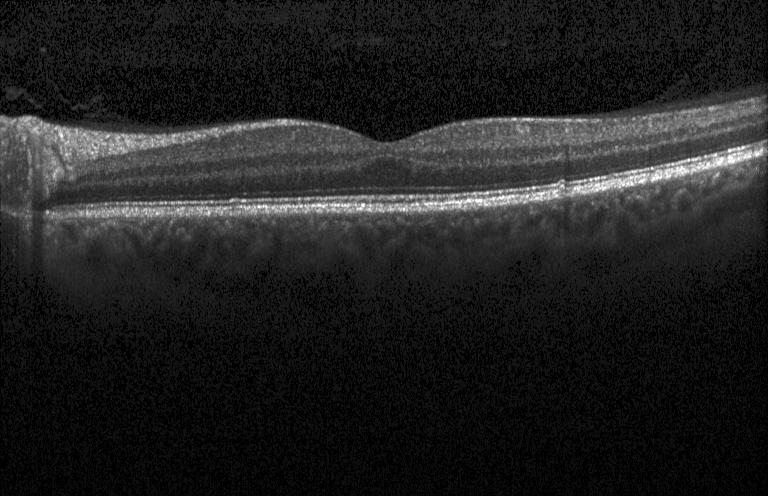 Horizontal scan through the fovea; acquired on a Heidelberg Spectralis; spectral-domain optical coherence tomography; OCT B-scan. Finding: no choroidal neovascularization, no diabetic macular edema, and no drusen.